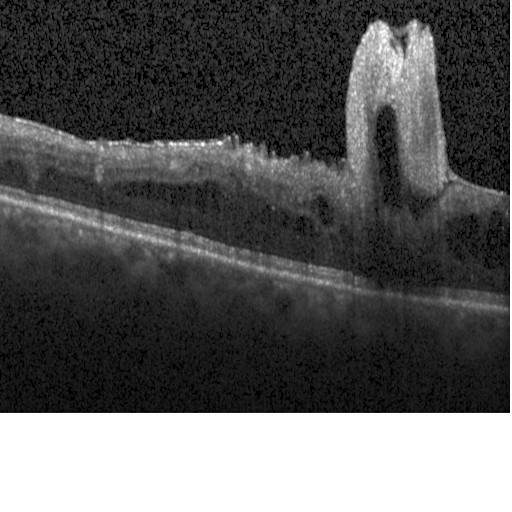 Impression: diabetic macular edema (DME).